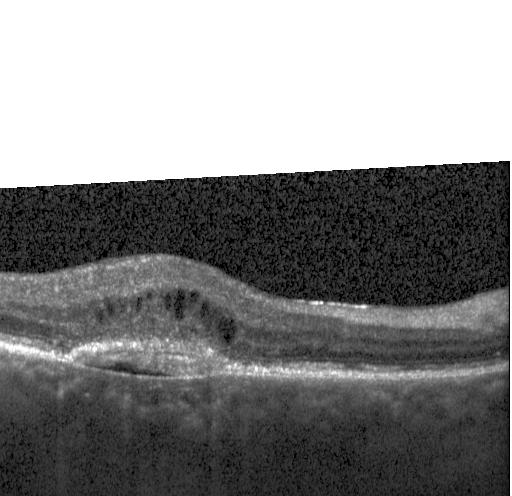
SD-OCT · fovea-centered · OCT B-scan
This B-scan demonstrates a choroidal neovascular membrane.